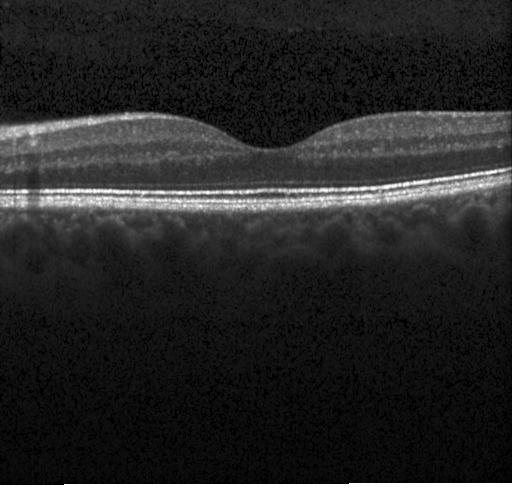

This B-scan demonstrates no choroidal neovascularization, diabetic macular edema, or drusen.